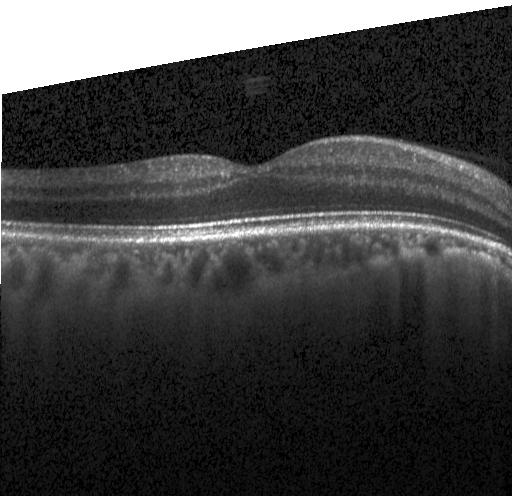 Through the macula · spectral-domain OCT · retinal OCT cross-section — Diagnosis: no evidence of choroidal neovascularization, diabetic macular edema, or drusen.